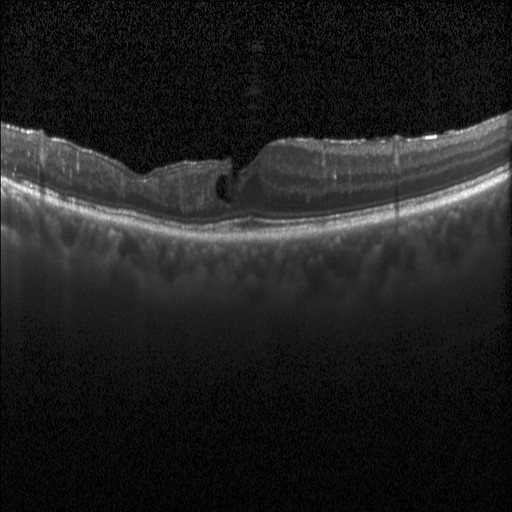 Instrument: Heidelberg Spectralis; SD-OCT; optical coherence tomography scan — Macular OCT: DME.